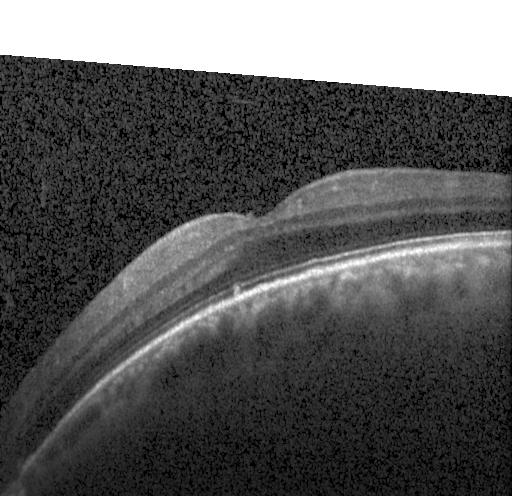

Finding: no evidence of choroidal neovascularization, diabetic macular edema, or drusen.